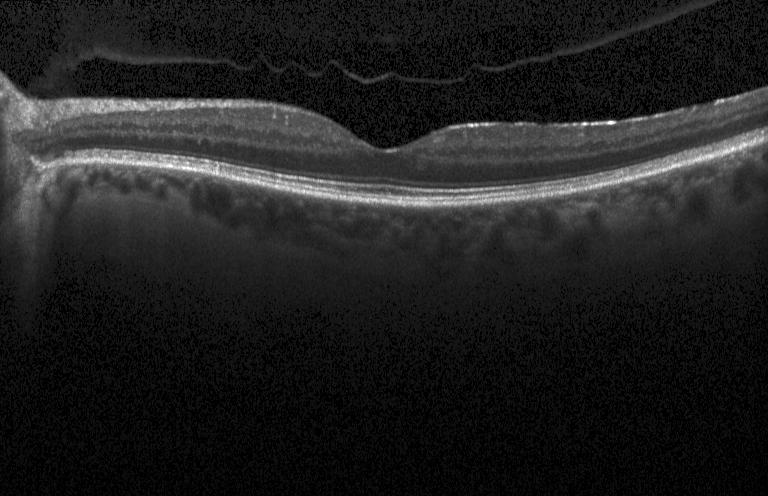
Acquired on a Heidelberg Spectralis · macular scan · retinal OCT B-scan · SD-OCT.
Diagnosis: neither choroidal neovascularization, diabetic macular edema, nor drusen.